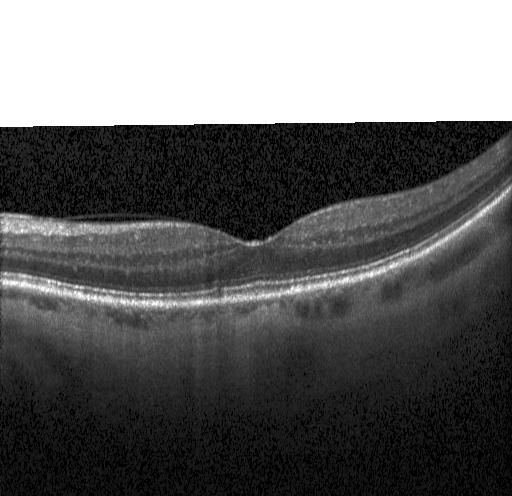

Spectral-domain OCT B-scan: no evidence of CNV, DME, or drusen.